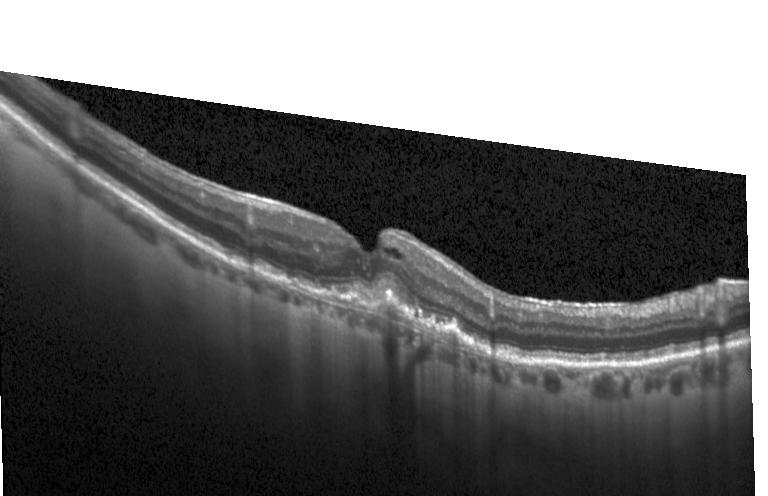 Retinal OCT cross-section showing choroidal neovascularization.